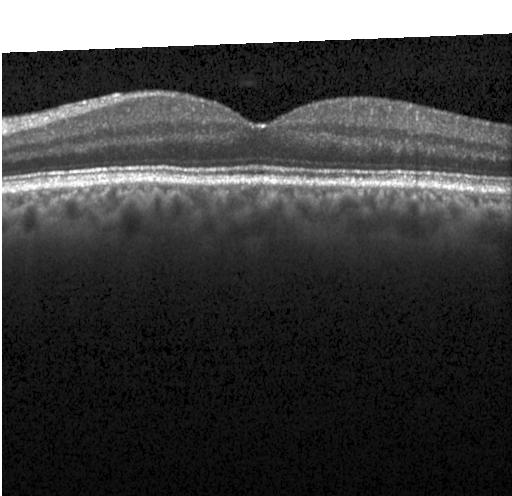
Retinal OCT cross-section; through the macula.
Diagnosis: no choroidal neovascularization, no diabetic macular edema, and no drusen.